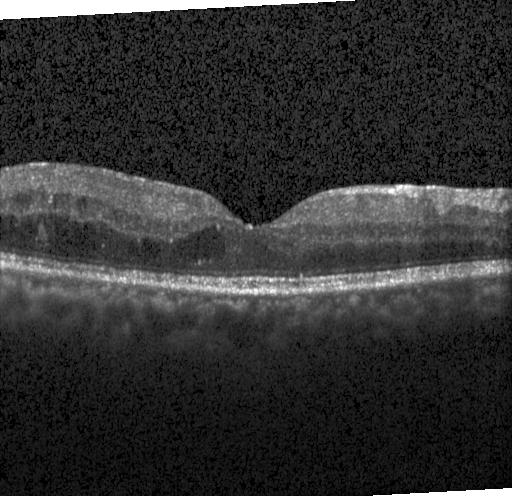 Optical coherence tomography scan, fovea-centered, SD-OCT. Macular OCT: diabetic macular edema.